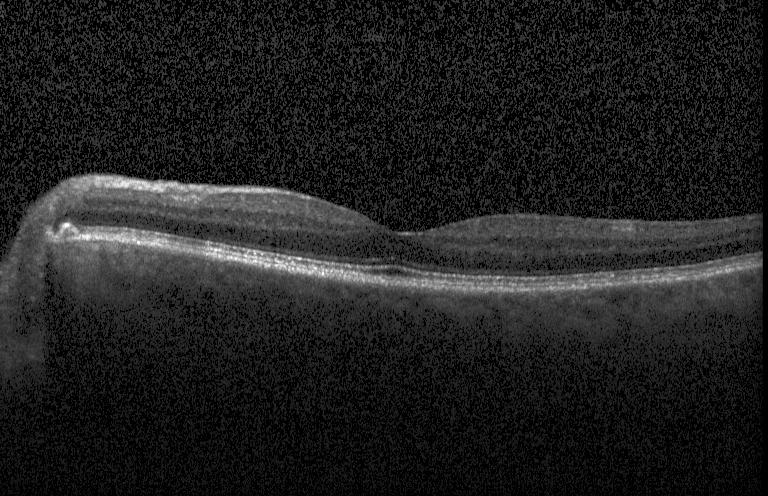

OCT B-scan
Diagnosis: neither CNV, DME, nor drusen.